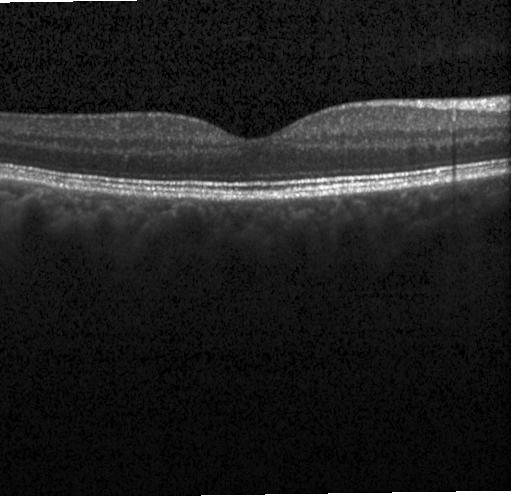

Spectral-domain optical coherence tomography. Centered on the fovea. Heidelberg Spectralis OCT system. Optical coherence tomography scan — No CNV, no DME, and no drusen.